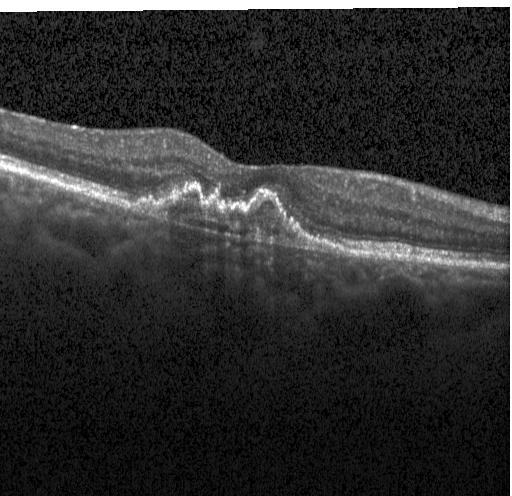

Impression: CNV.